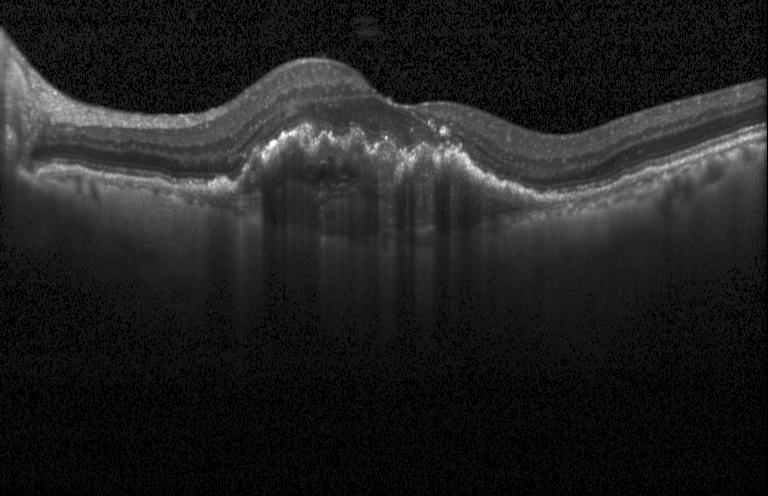 Heidelberg Spectralis, optical coherence tomography B-scan, centered on the fovea — Diagnosis: a choroidal neovascular membrane.